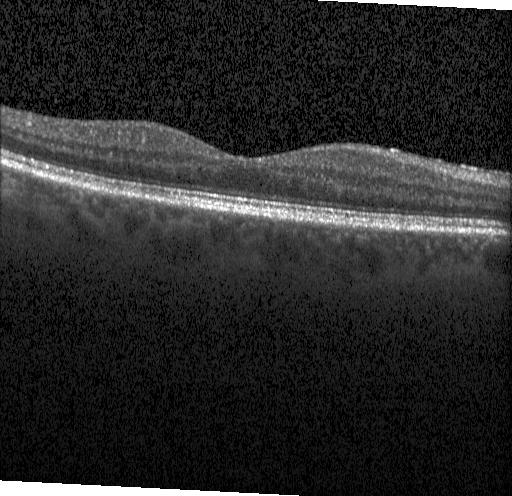 Finding: neither CNV, DME, nor drusen.